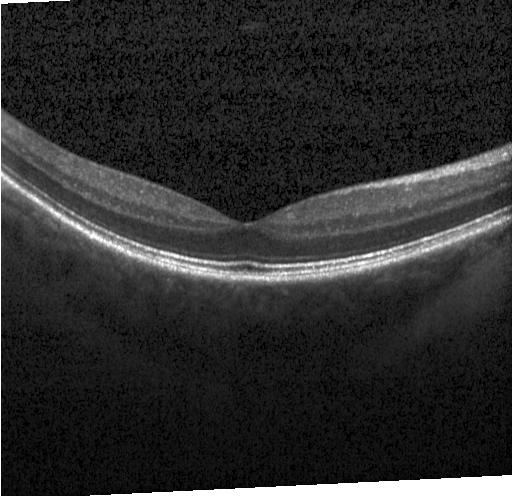
Retinal OCT cross-section
Diagnosis: no evidence of choroidal neovascularization, diabetic macular edema, or drusen.